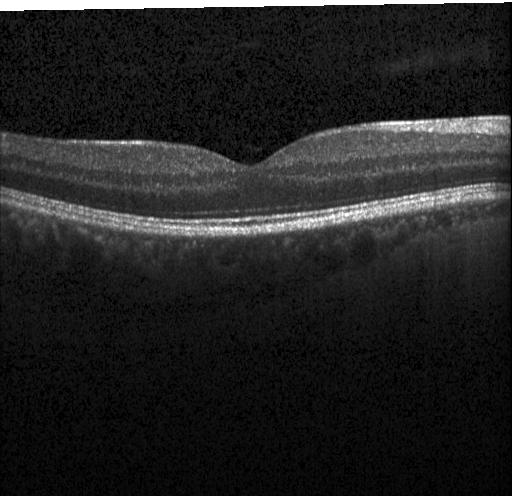 Heidelberg Spectralis. OCT B-scan
This B-scan demonstrates no choroidal neovascularization, no diabetic macular edema, and no drusen.